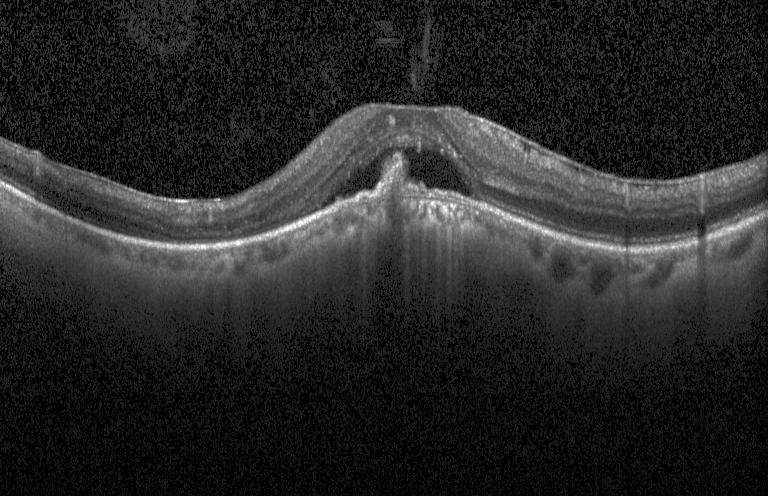

Impression: a choroidal neovascular membrane.